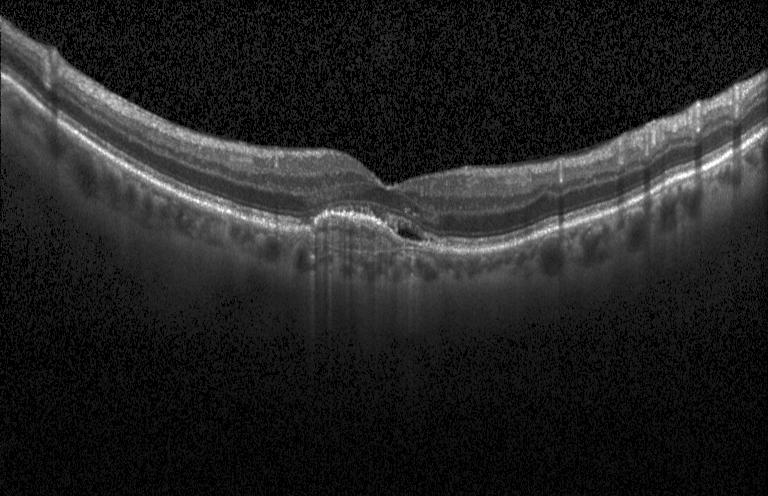 SD-OCT, optical coherence tomography B-scan — Choroidal neovascularization.